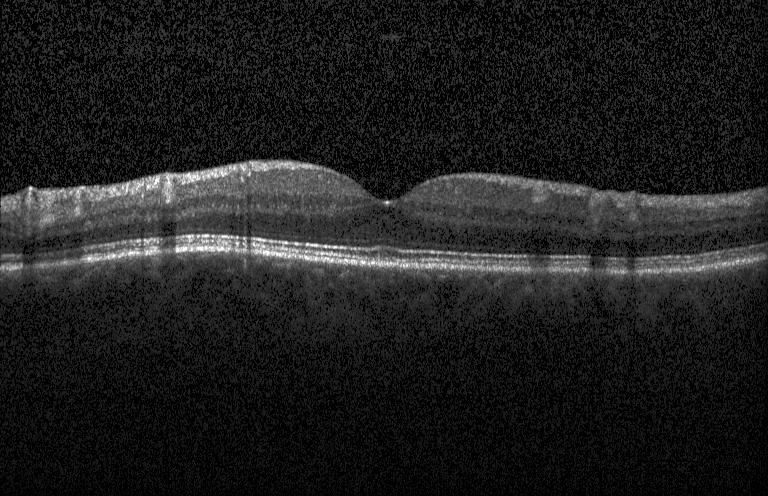
Macular OCT demonstrating no CNV, DME, or drusen.